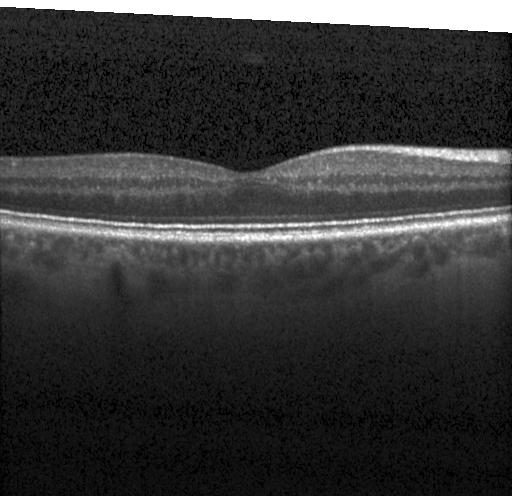
Assessment: neither choroidal neovascularization, diabetic macular edema, nor drusen.